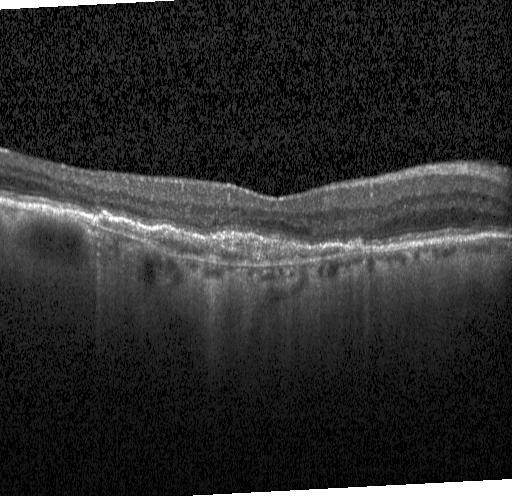

This B-scan demonstrates choroidal neovascularization (CNV).